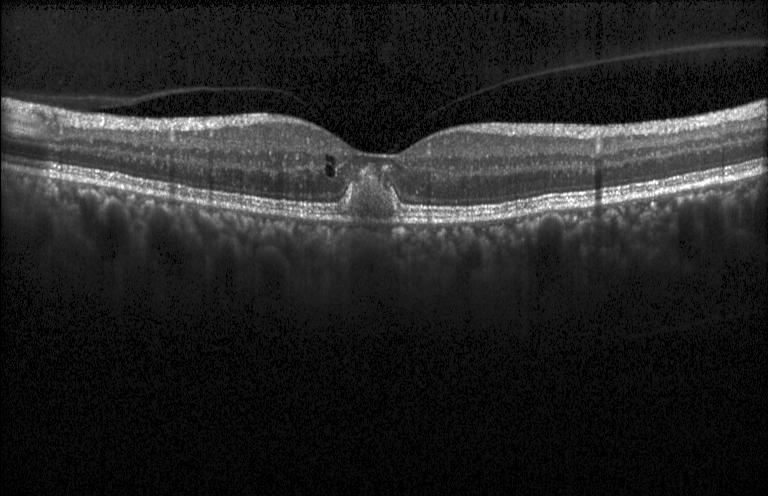

Centered on the fovea, SD-OCT, retinal OCT cross-section — Choroidal neovascularization (CNV).